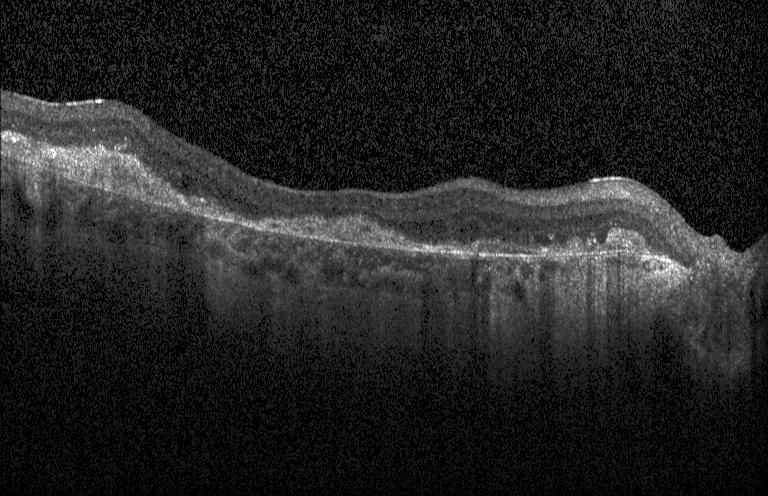

Acquired on a Heidelberg Spectralis; optical coherence tomography B-scan; SD-OCT; fovea-centered — This B-scan demonstrates CNV.